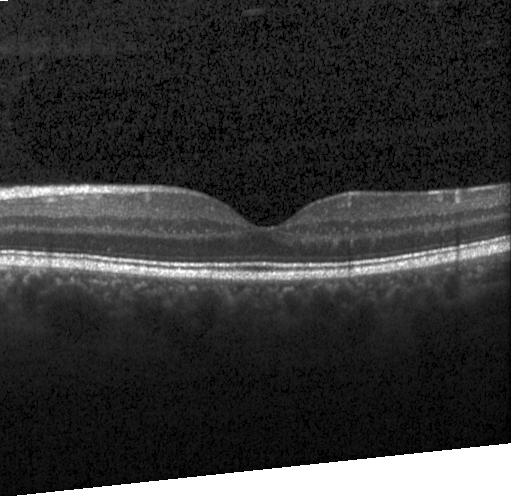 Heidelberg Spectralis; through the macula; spectral-domain optical coherence tomography; optical coherence tomography scan
Dx: no evidence of choroidal neovascularization, diabetic macular edema, or drusen.